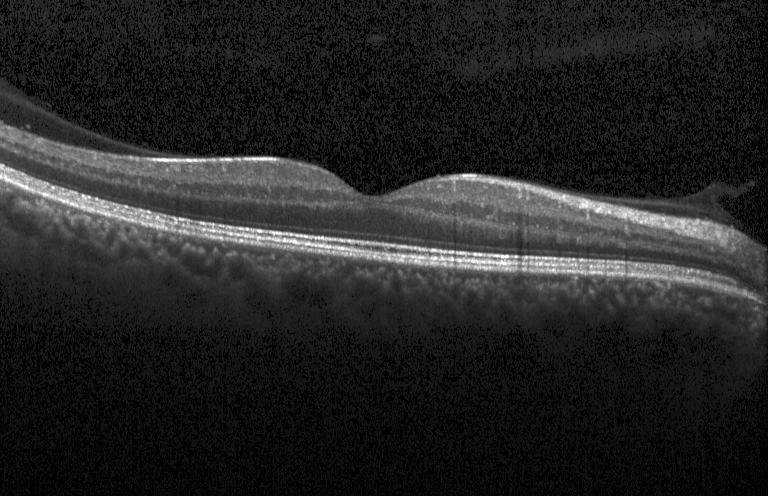 This B-scan demonstrates neither CNV, DME, nor drusen.